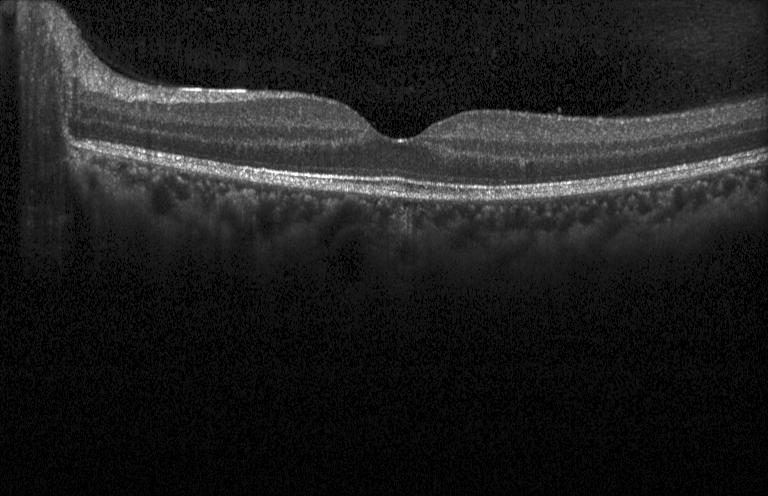

Macular OCT demonstrating no choroidal neovascularization, diabetic macular edema, or drusen.